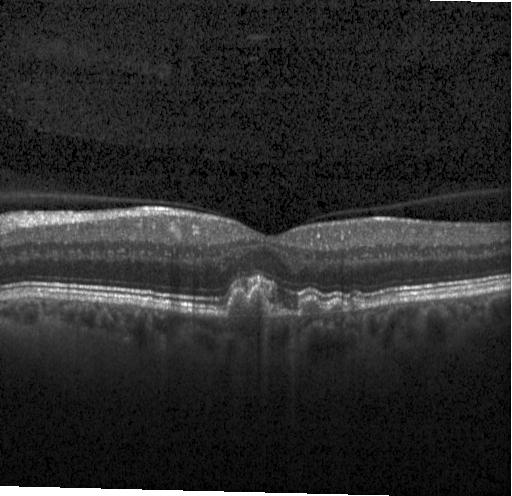 This B-scan demonstrates drusen.